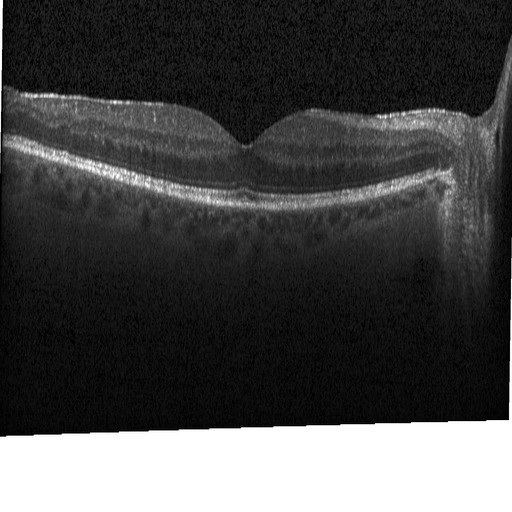
Fovea-centered. Spectral-domain optical coherence tomography. Retinal OCT cross-section. Heidelberg Spectralis OCT system. Finding: diabetic macular edema.